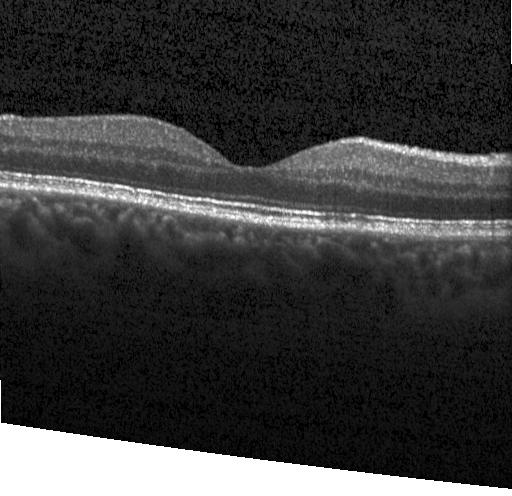 OCT finding: neither choroidal neovascularization, diabetic macular edema, nor drusen.